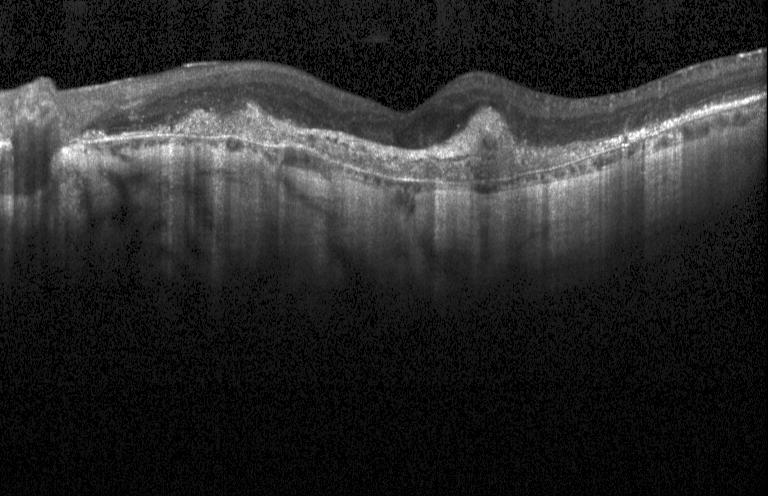 Macular OCT demonstrating a choroidal neovascular membrane.